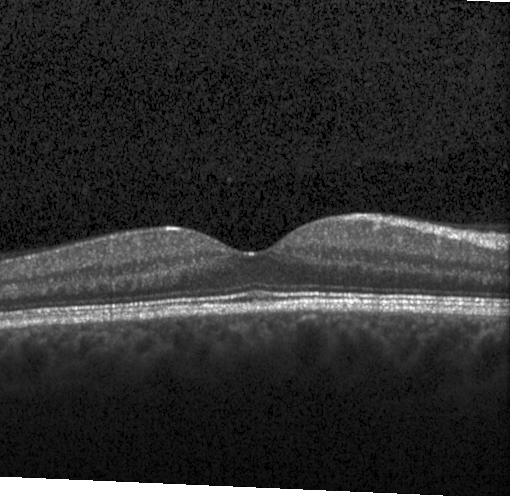
Fovea-centered, retinal OCT B-scan. Impression: no choroidal neovascularization, diabetic macular edema, or drusen.